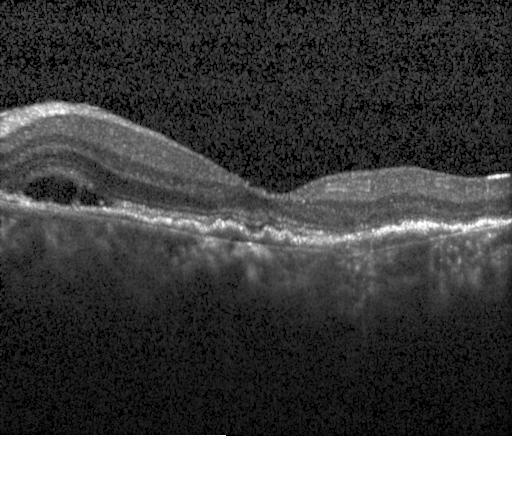

Retinal OCT cross-section showing choroidal neovascularization.